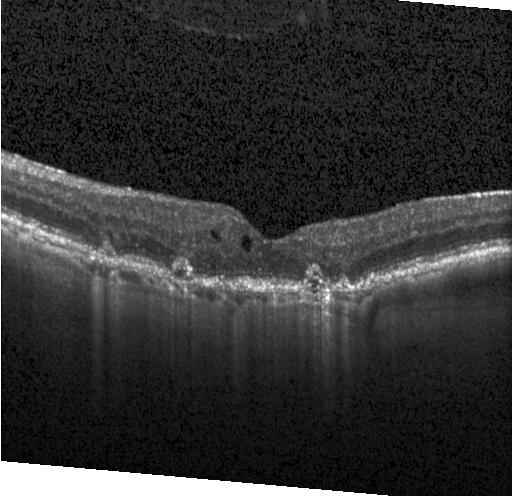 Spectral-domain OCT, retinal OCT B-scan, acquired on a Heidelberg Spectralis.
Assessment: a choroidal neovascular membrane.